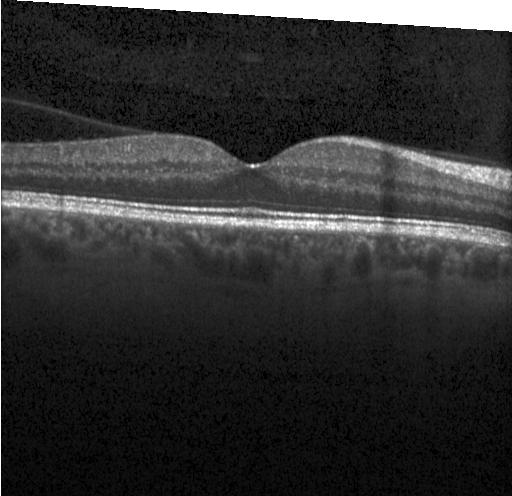 Acquired on a Heidelberg Spectralis. Optical coherence tomography scan. Fovea-centered
Finding: neither choroidal neovascularization, diabetic macular edema, nor drusen.